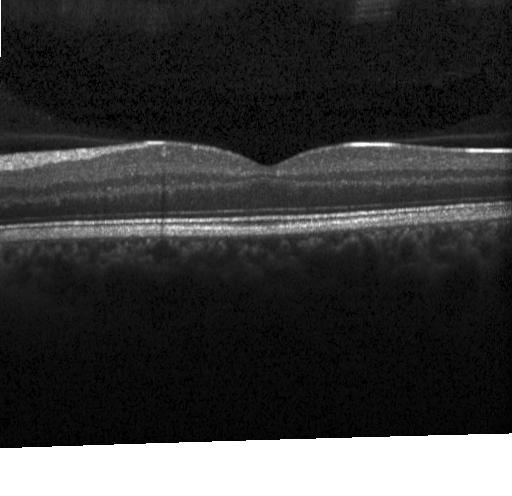 Impression: no choroidal neovascularization, no diabetic macular edema, and no drusen.